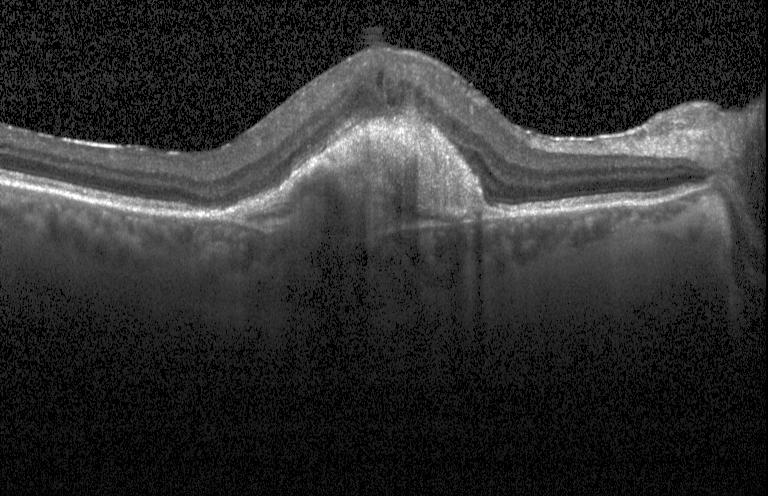
Heidelberg Spectralis · OCT B-scan.
Finding: choroidal neovascularization.